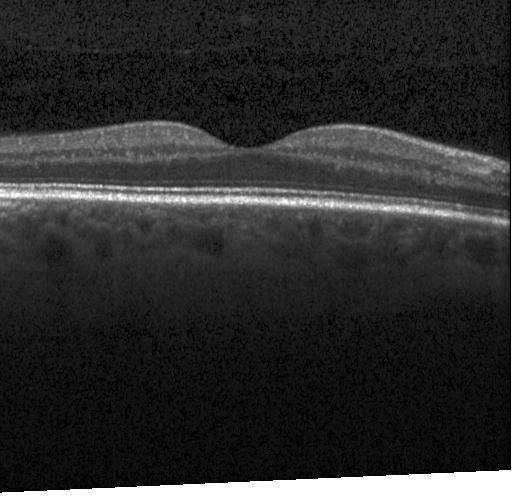 OCT line scan
Diagnosis: no CNV, DME, or drusen.